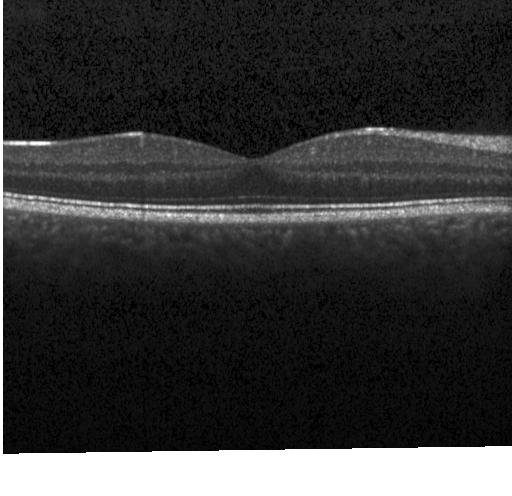 Retinal OCT cross-section showing no evidence of CNV, DME, or drusen.